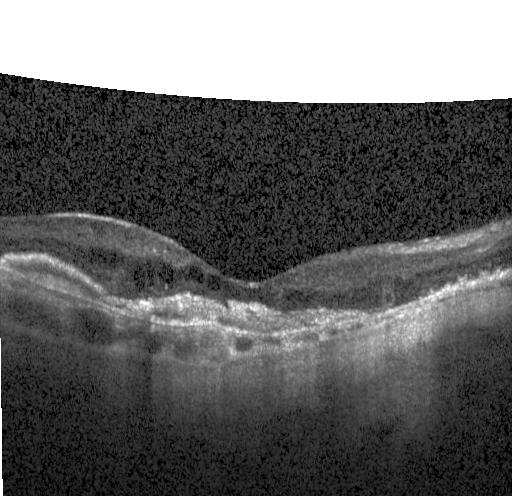

Acquired on a Heidelberg Spectralis, retinal OCT B-scan — The scan shows choroidal neovascularization (CNV).